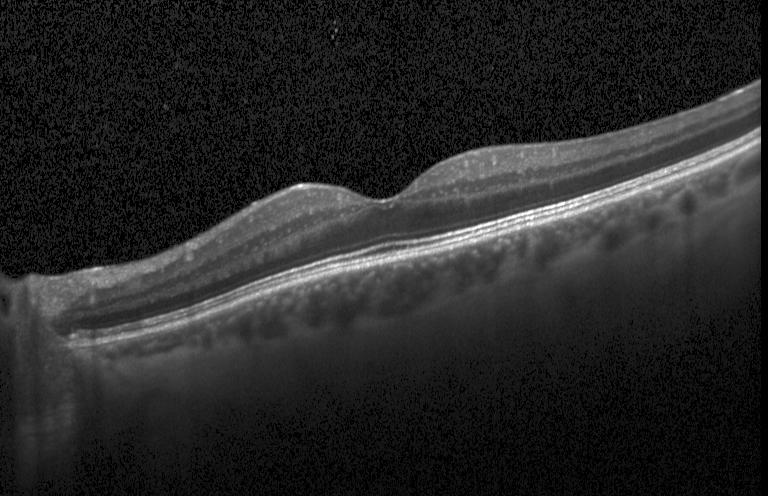

Spectral-domain OCT B-scan: neither choroidal neovascularization, diabetic macular edema, nor drusen.